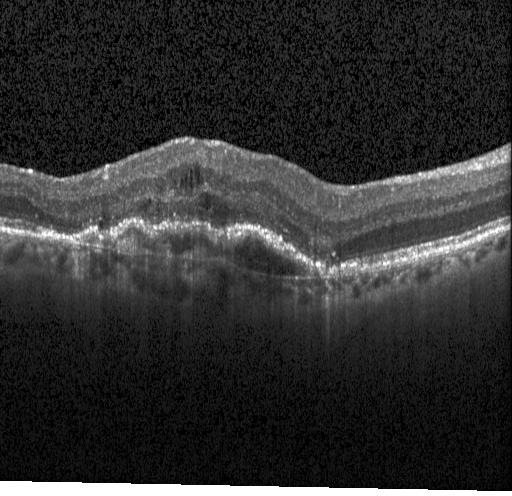
A choroidal neovascular membrane.